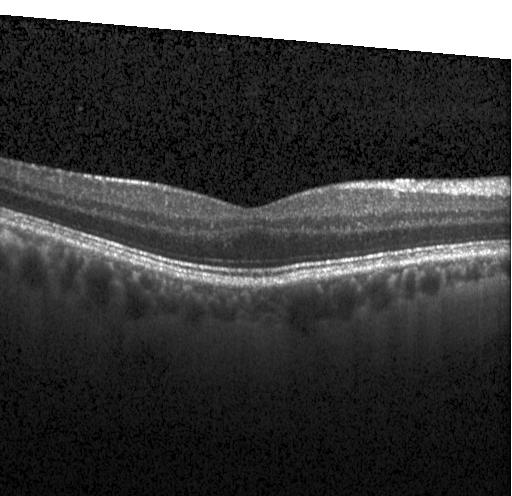

Centered on the fovea. Retinal OCT B-scan. Spectral-domain optical coherence tomography. Heidelberg Spectralis OCT system.
Assessment: no CNV, DME, or drusen.